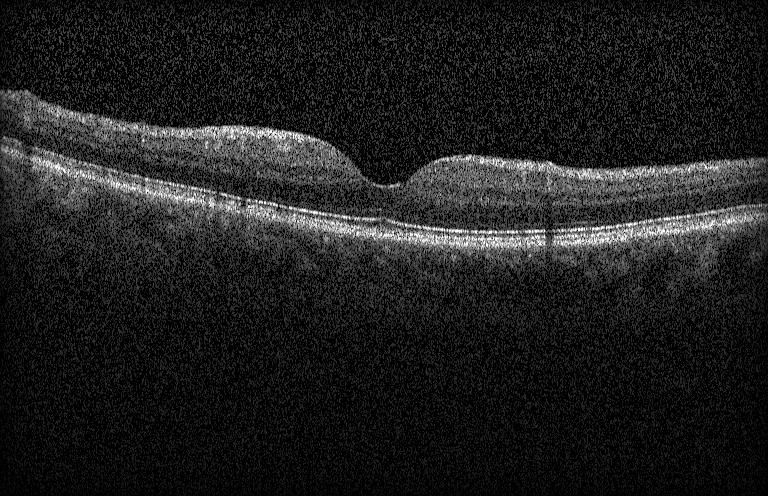 OCT B-scan, fovea-centered.
OCT finding: no choroidal neovascularization, no diabetic macular edema, and no drusen.